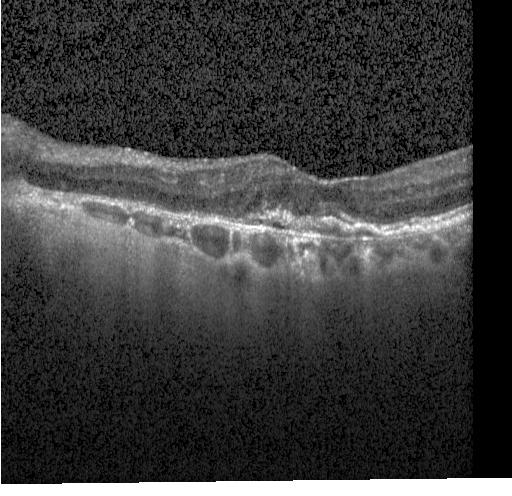
Spectral-domain OCT · Heidelberg Spectralis · fovea-centered · retinal OCT cross-section. Assessment: a choroidal neovascular membrane.